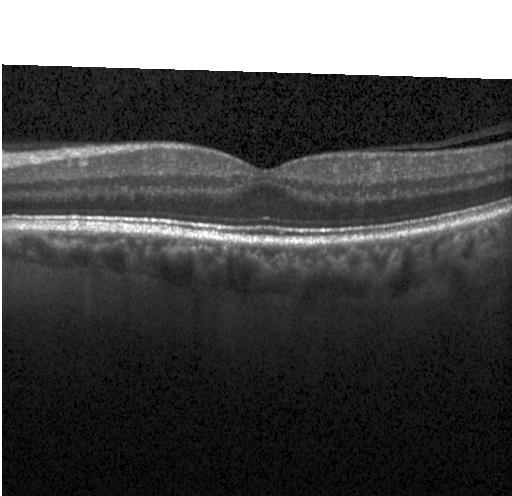

Impression: no choroidal neovascularization, no diabetic macular edema, and no drusen.